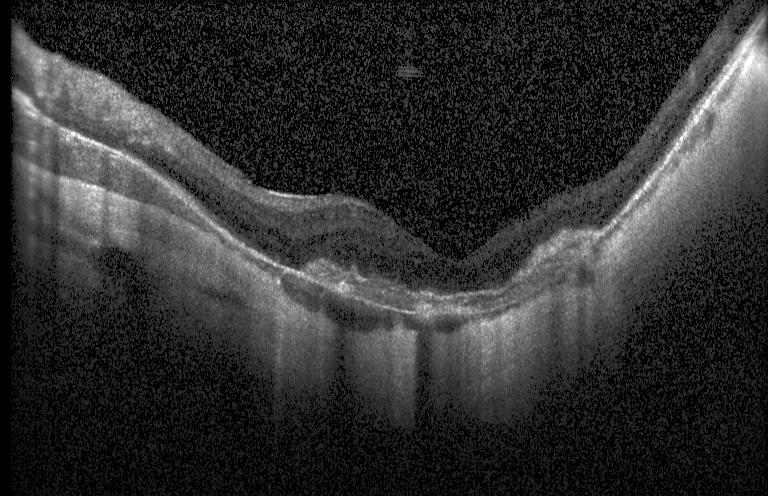
The scan shows a choroidal neovascular membrane.